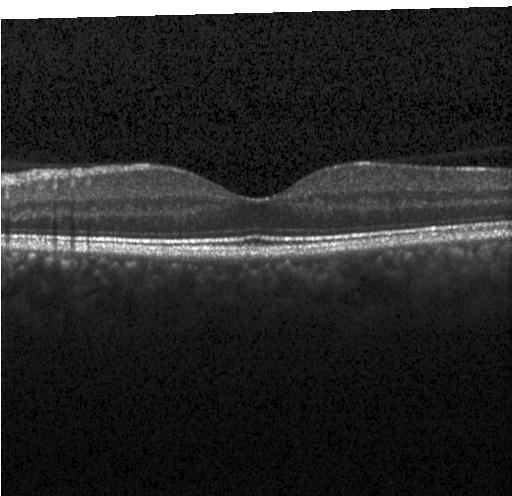
Retinal OCT B-scan, Heidelberg Spectralis OCT system
Diagnosis: no CNV, DME, or drusen.